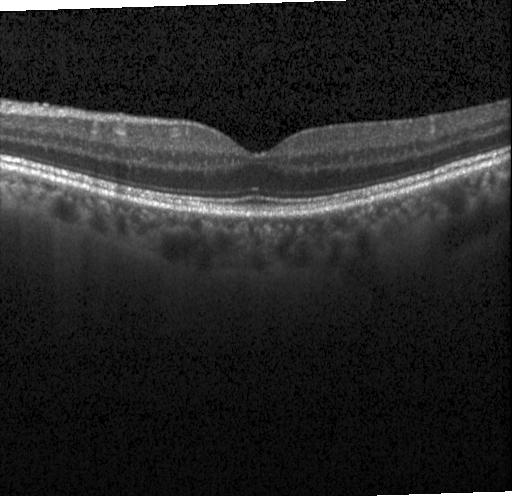
Retinal OCT cross-section. Spectral-domain optical coherence tomography. Through the macula. Heidelberg Spectralis.
This B-scan demonstrates no evidence of choroidal neovascularization, diabetic macular edema, or drusen.